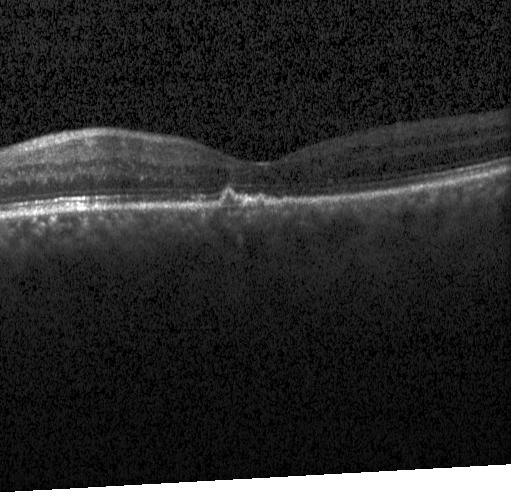 Instrument: Heidelberg Spectralis; optical coherence tomography B-scan
The scan shows multiple drusen.